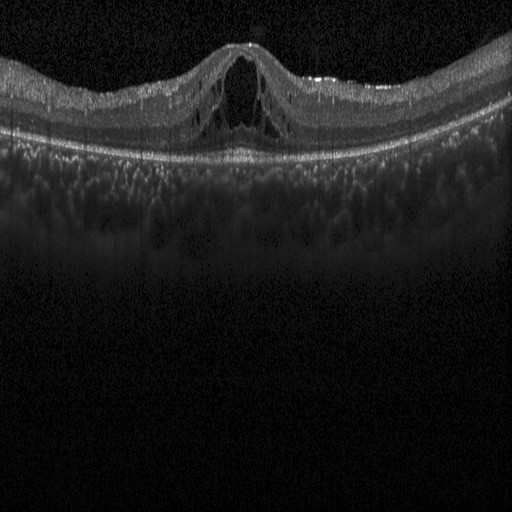 Macular scan · retinal OCT B-scan.
Macular OCT: DME.